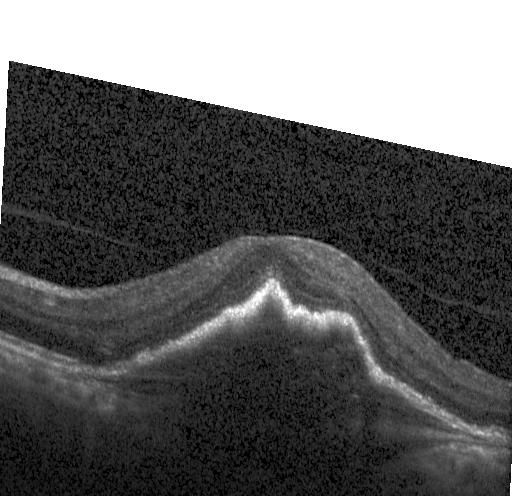 Macular OCT demonstrating choroidal neovascularization.